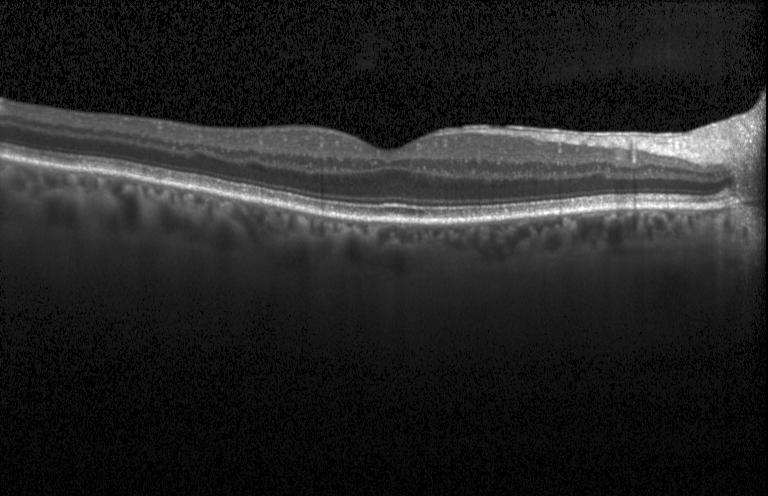 OCT line scan · fovea-centered · Heidelberg Spectralis OCT system.
The scan shows no evidence of choroidal neovascularization, diabetic macular edema, or drusen.